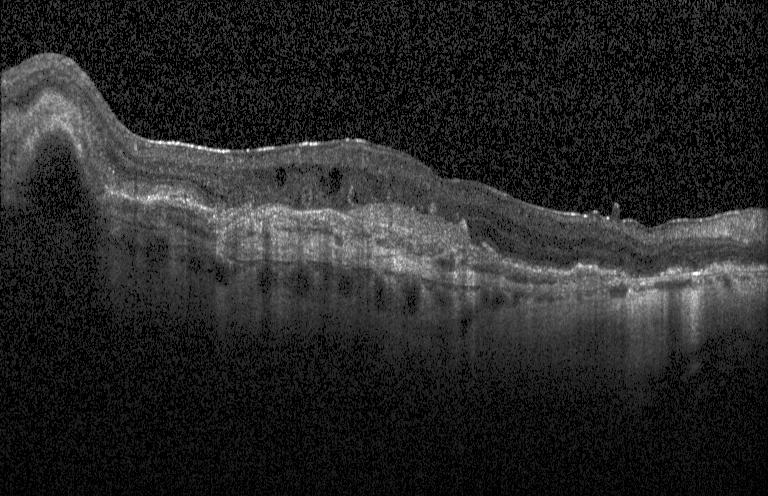
Fovea-centered · optical coherence tomography scan. Diagnosis: choroidal neovascularization.